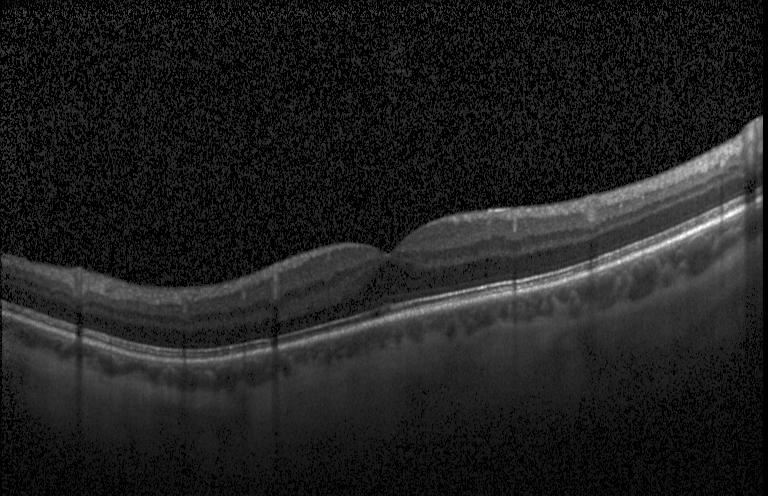
Horizontal scan through the fovea; Heidelberg Spectralis; OCT line scan.
The scan shows no choroidal neovascularization, no diabetic macular edema, and no drusen.